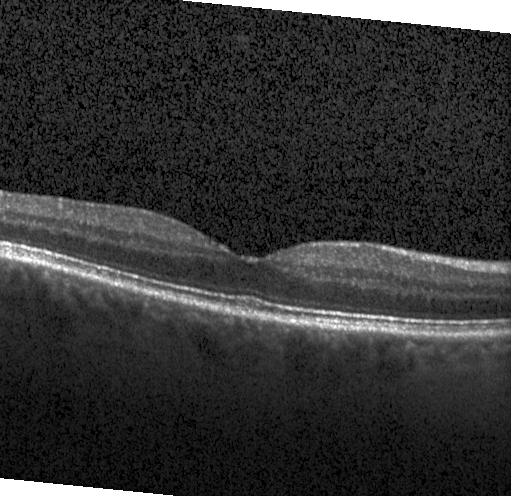 Retinal OCT B-scan · spectral-domain optical coherence tomography · instrument: Heidelberg Spectralis — Macular OCT: no choroidal neovascularization, diabetic macular edema, or drusen.